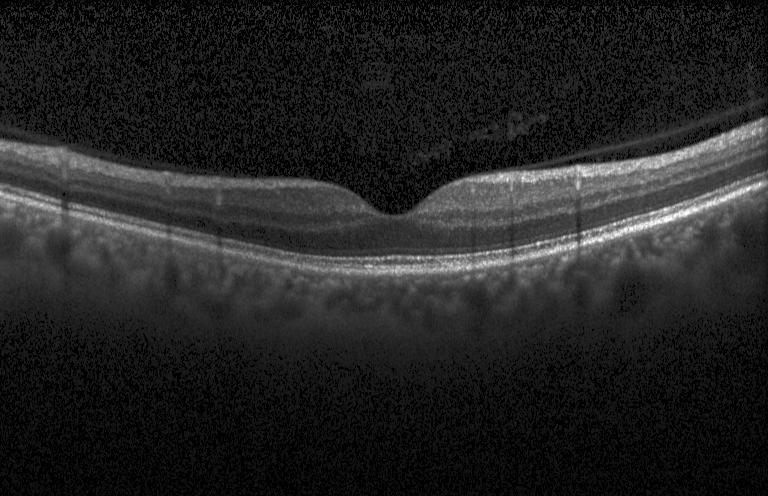
Impression: no choroidal neovascularization, no diabetic macular edema, and no drusen.